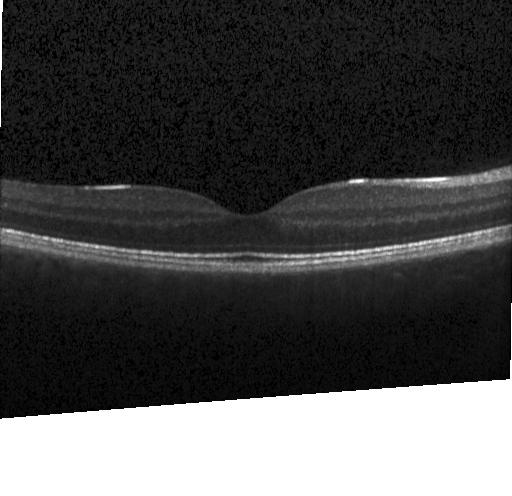 Spectral-domain OCT B-scan: no choroidal neovascularization, diabetic macular edema, or drusen.